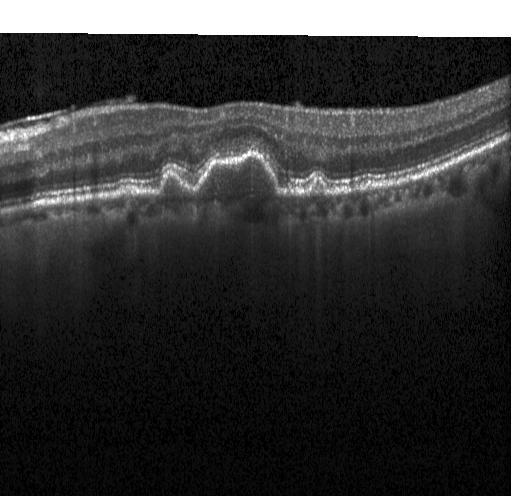

Finding: a choroidal neovascular membrane.